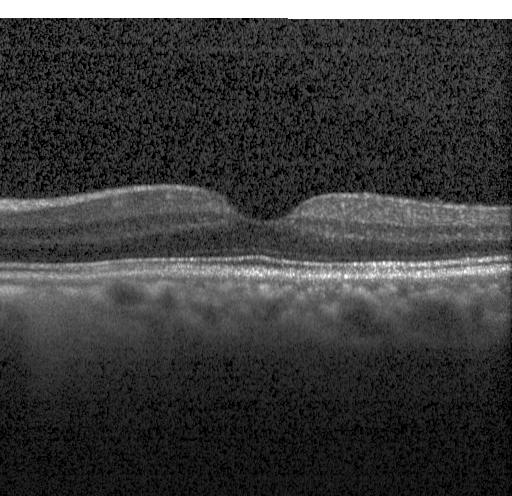
Heidelberg Spectralis; OCT B-scan — Impression: no evidence of choroidal neovascularization, diabetic macular edema, or drusen.